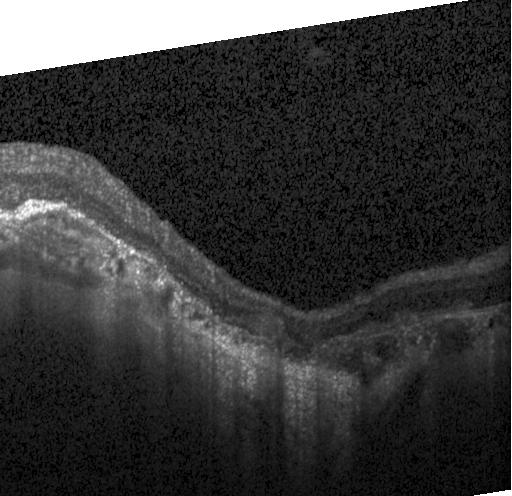
Acquired on a Heidelberg Spectralis · retinal OCT B-scan. A choroidal neovascular membrane.